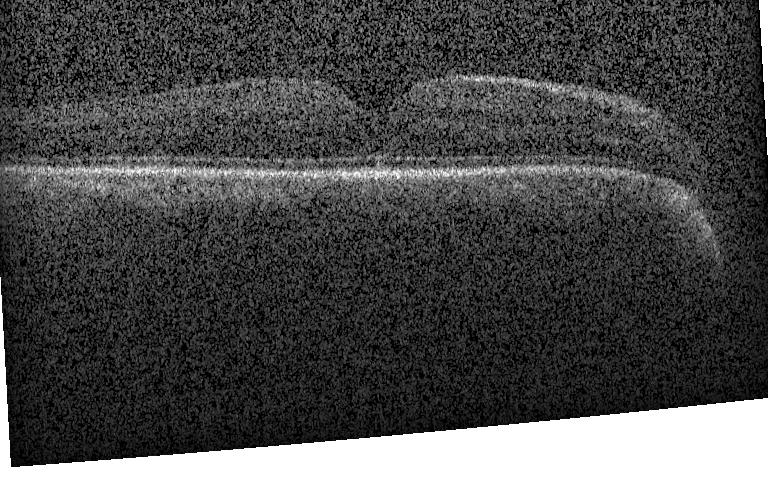
Diagnosis: no evidence of choroidal neovascularization, diabetic macular edema, or drusen.